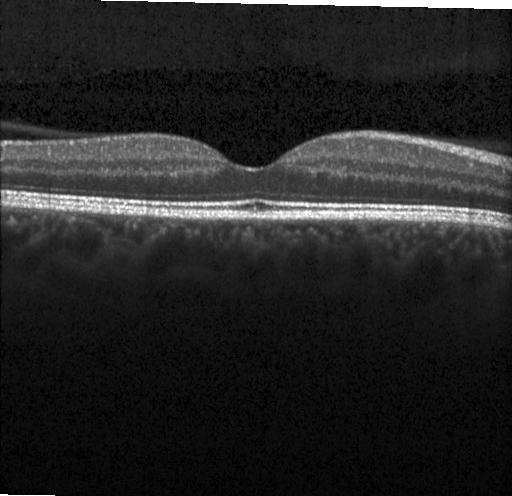
OCT B-scan
Finding: no CNV, DME, or drusen.